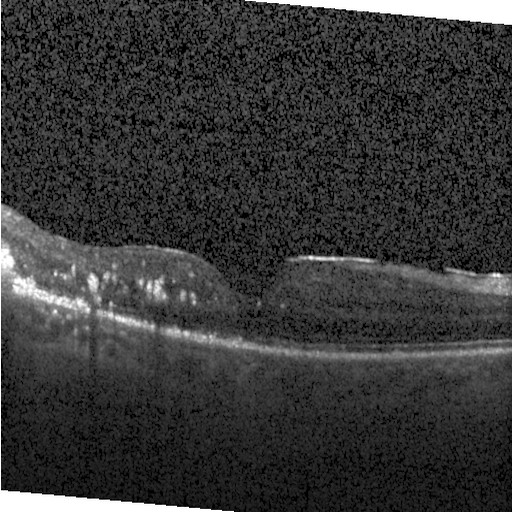 Spectral-domain OCT B-scan: DME.